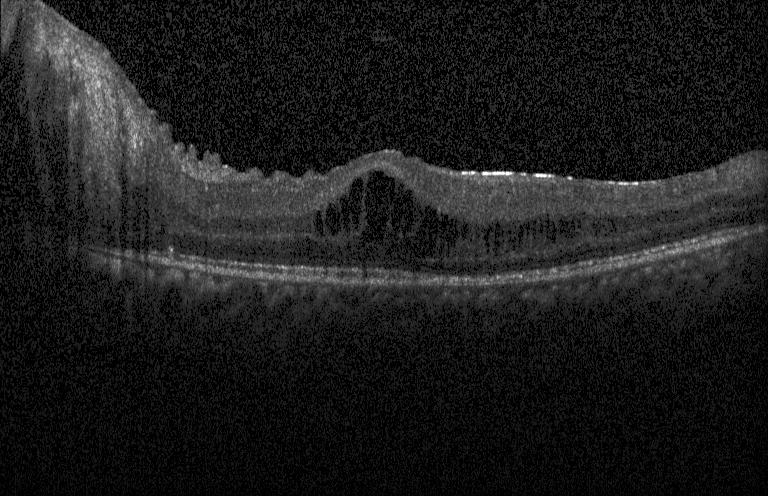 Optical coherence tomography B-scan, spectral-domain OCT, acquired on a Heidelberg Spectralis, through the macula.
Macular OCT: DME.